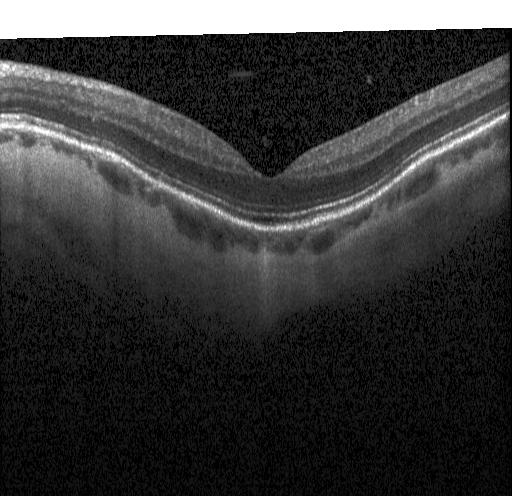 Optical coherence tomography B-scan; spectral-domain OCT; through the macula — Impression: no evidence of choroidal neovascularization, diabetic macular edema, or drusen.